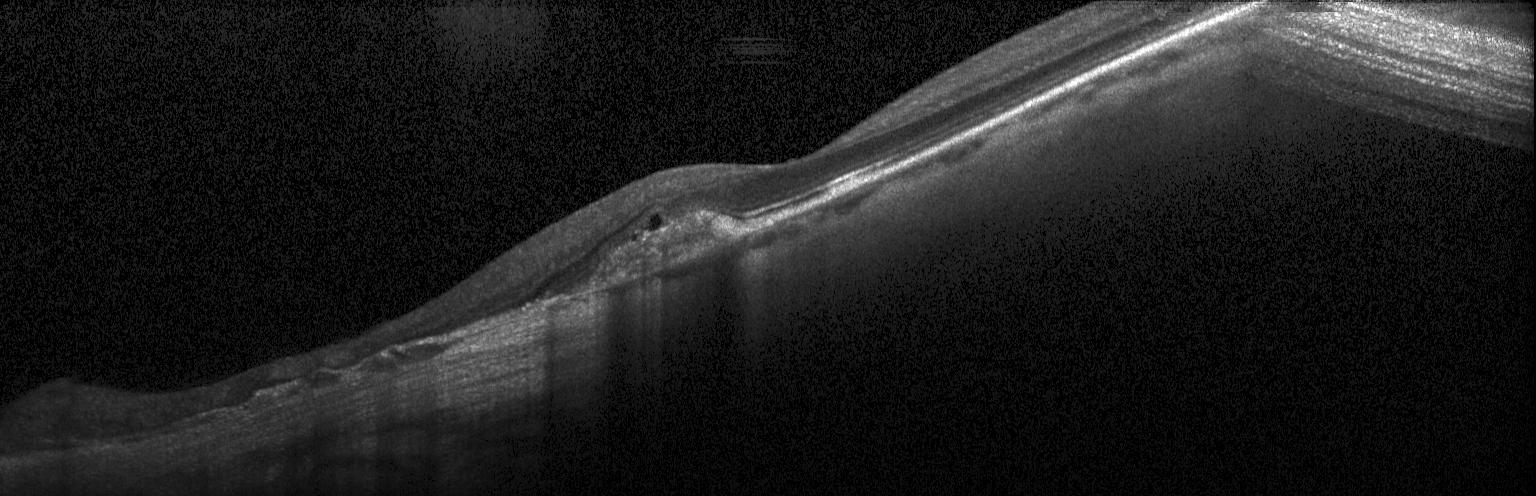
Impression: a choroidal neovascular membrane.